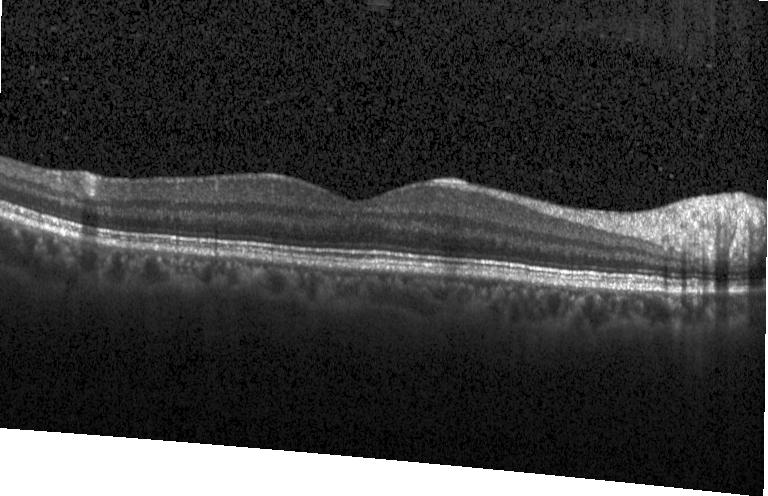 OCT B-scan showing neither choroidal neovascularization, diabetic macular edema, nor drusen.